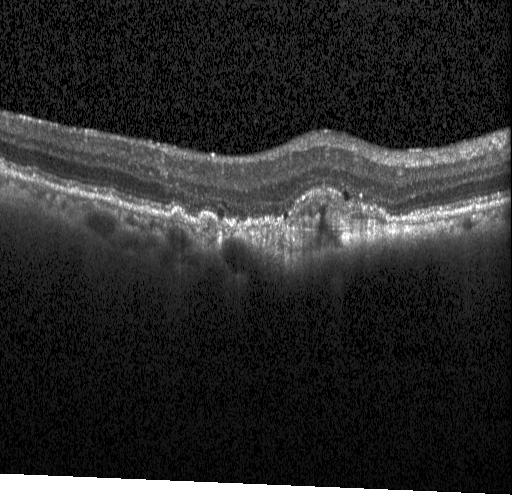 OCT B-scan showing a choroidal neovascular membrane.